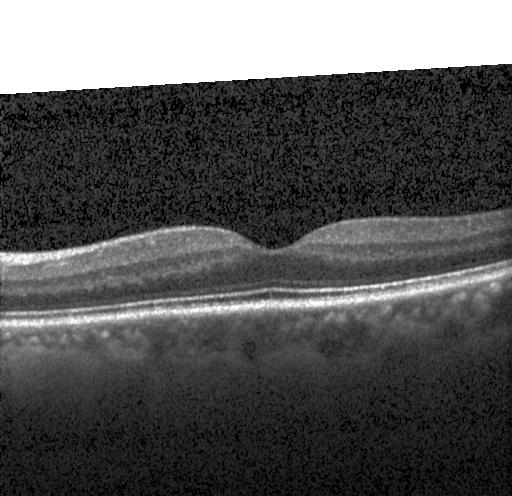

Impression: no evidence of choroidal neovascularization, diabetic macular edema, or drusen.